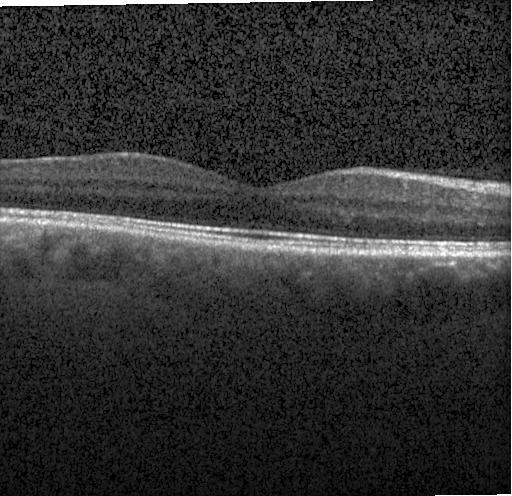

Macular OCT demonstrating no choroidal neovascularization, no diabetic macular edema, and no drusen.